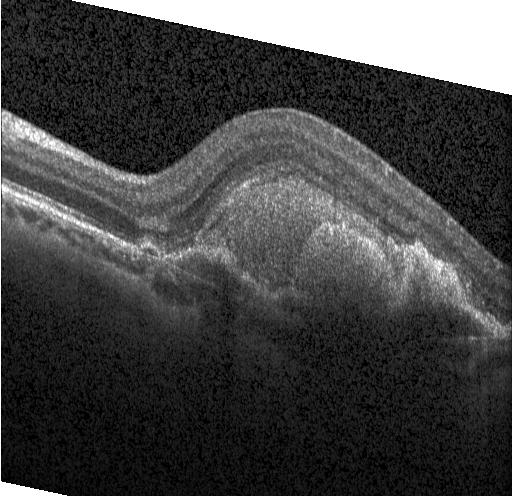

Retinal OCT cross-section. Macular scan. This B-scan demonstrates choroidal neovascularization.